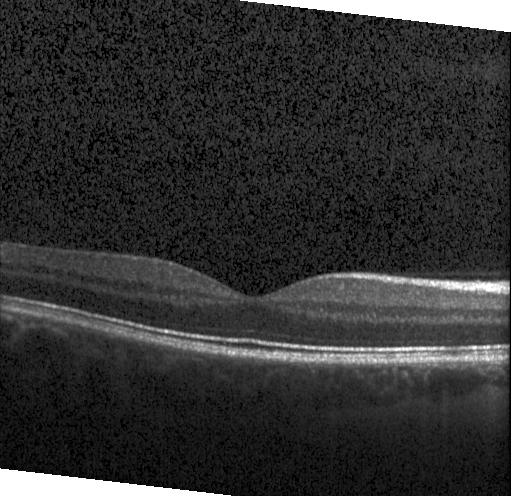 Dx: no evidence of choroidal neovascularization, diabetic macular edema, or drusen.